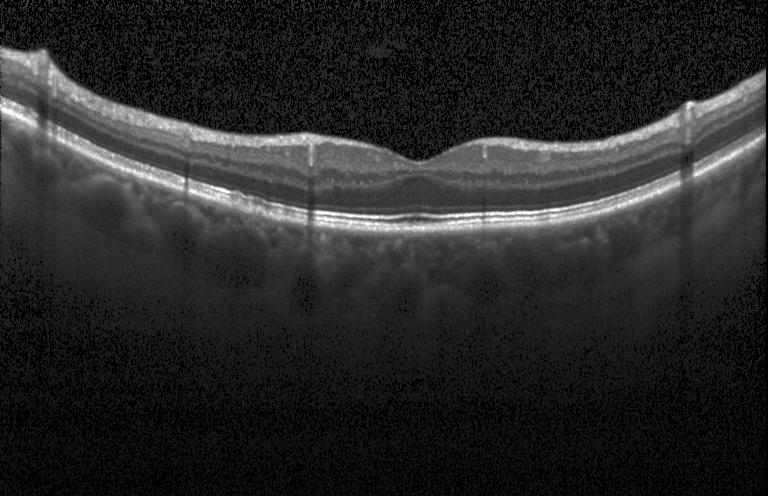

No choroidal neovascularization, no diabetic macular edema, and no drusen.